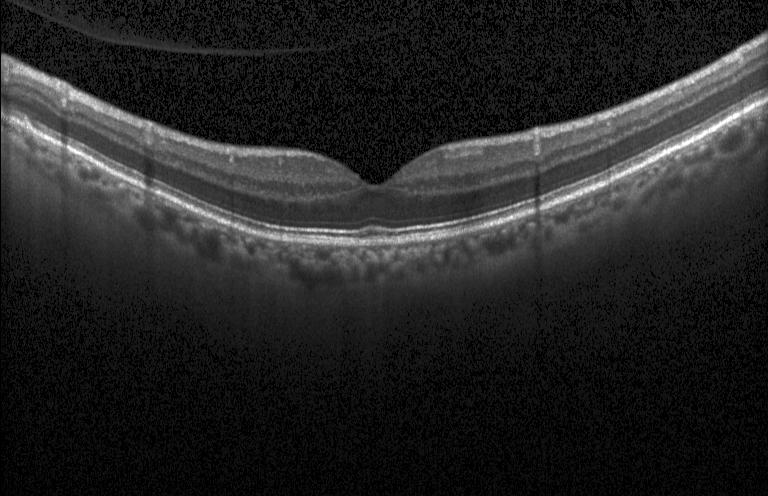 Assessment: neither CNV, DME, nor drusen.